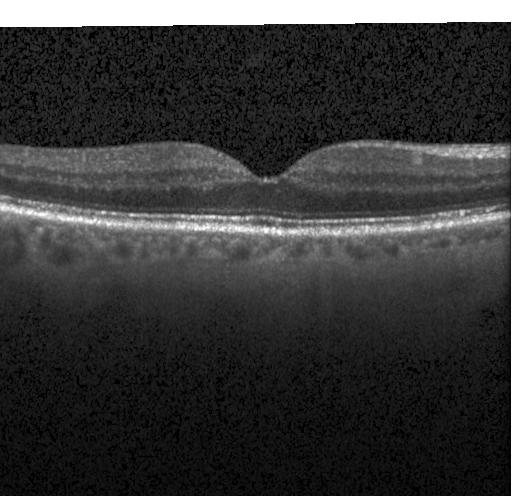 Heidelberg Spectralis · SD-OCT · horizontal scan through the fovea · retinal OCT cross-section
OCT finding: no evidence of choroidal neovascularization, diabetic macular edema, or drusen.